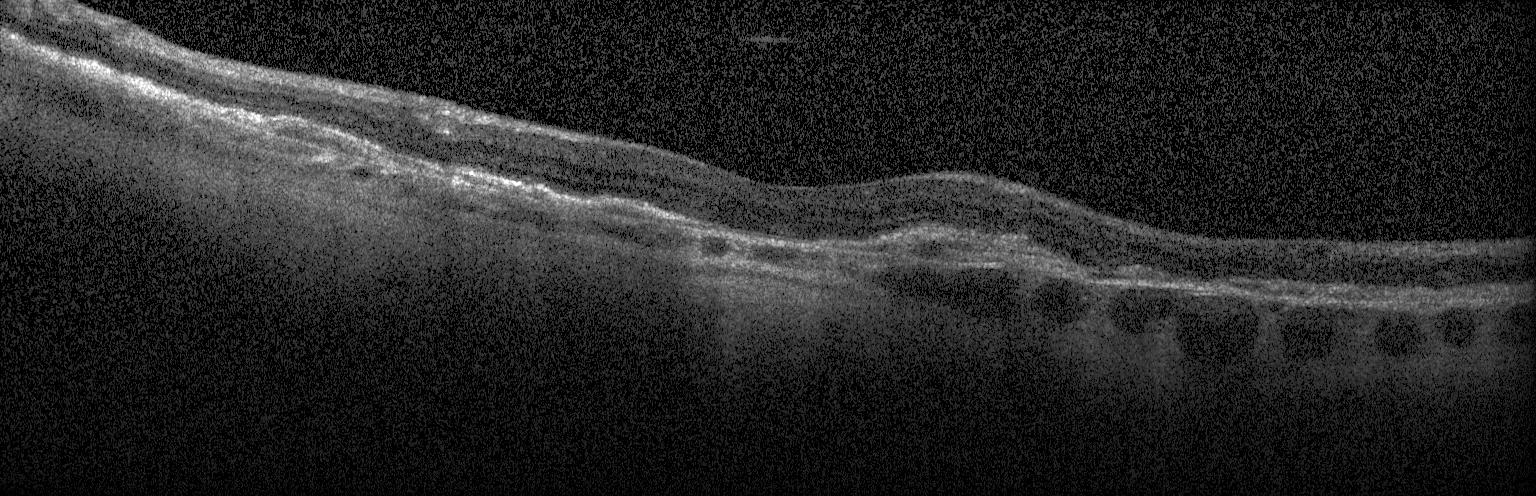

Optical coherence tomography scan — Dx: CNV.